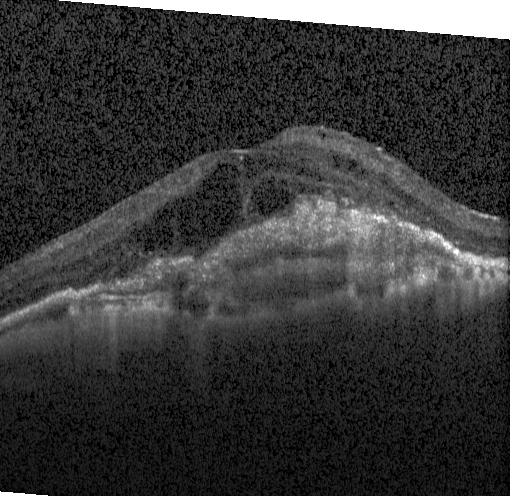
The scan shows CNV.